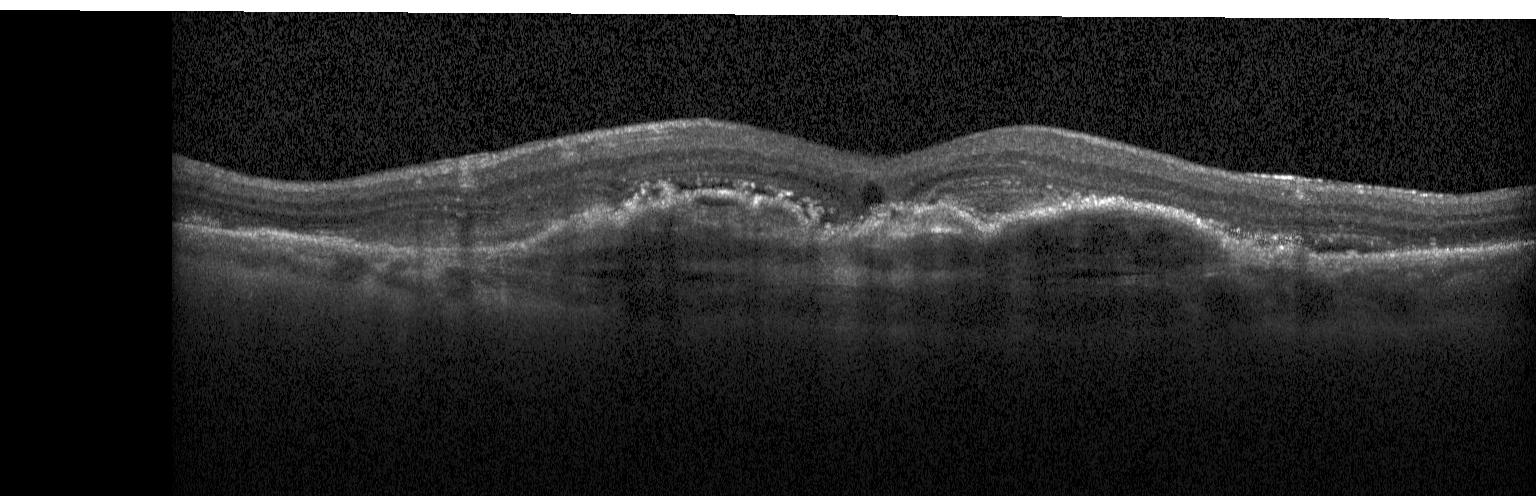
OCT finding: CNV.